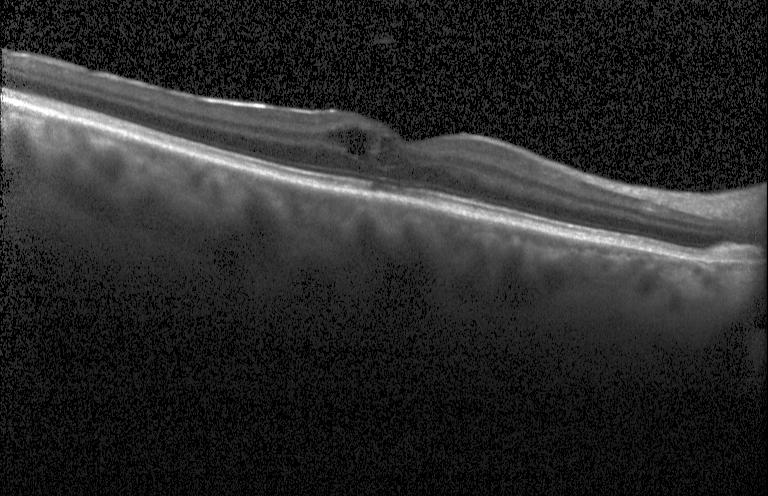
SD-OCT; optical coherence tomography B-scan
Diabetic macular edema.